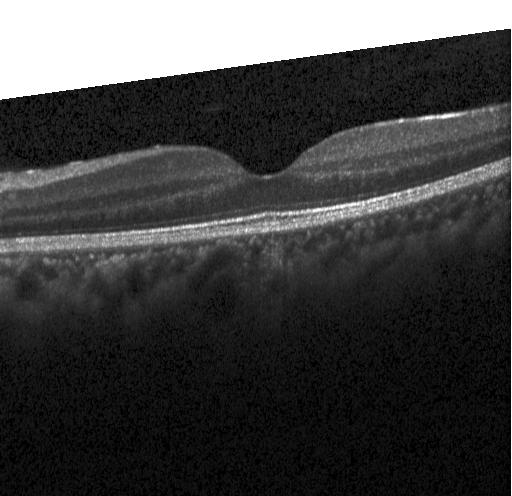 Finding: no CNV, DME, or drusen.